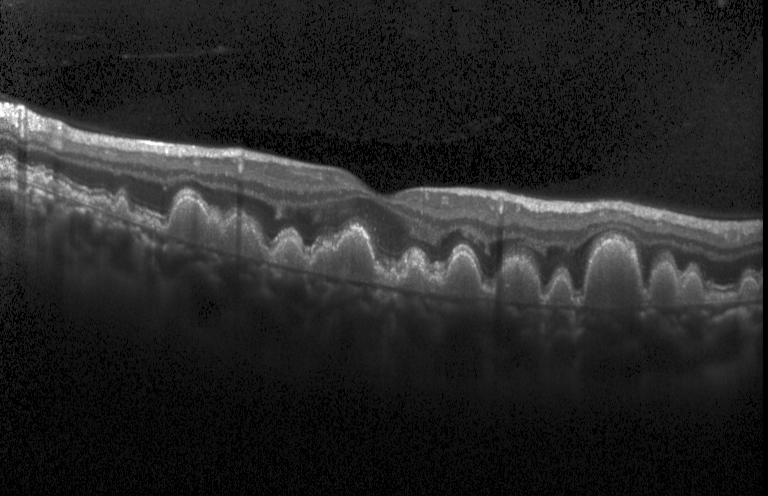

Spectral-domain optical coherence tomography. OCT B-scan. Instrument: Heidelberg Spectralis. Fovea-centered. Finding: multiple drusen.